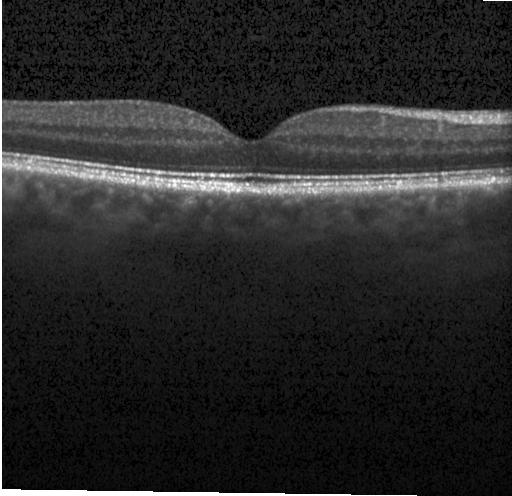
Macular scan, Heidelberg Spectralis OCT system, retinal OCT cross-section, SD-OCT
OCT finding: no choroidal neovascularization, diabetic macular edema, or drusen.